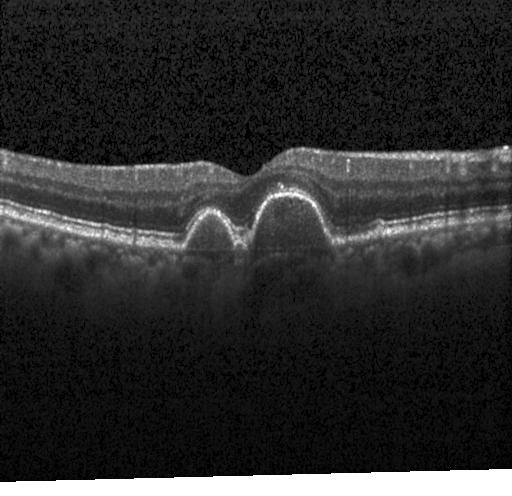
OCT finding: multiple drusen.